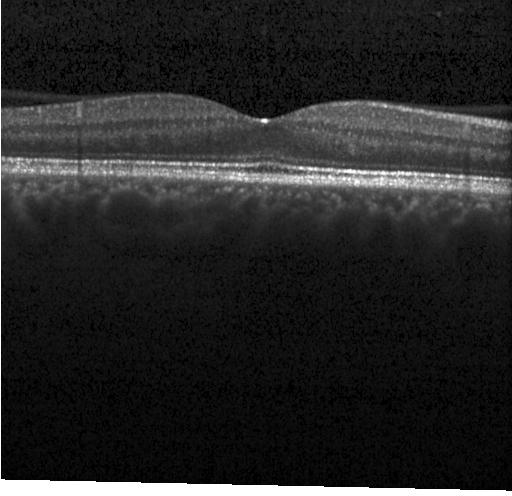
Spectral-domain OCT; OCT B-scan — Diagnosis: no choroidal neovascularization, no diabetic macular edema, and no drusen.